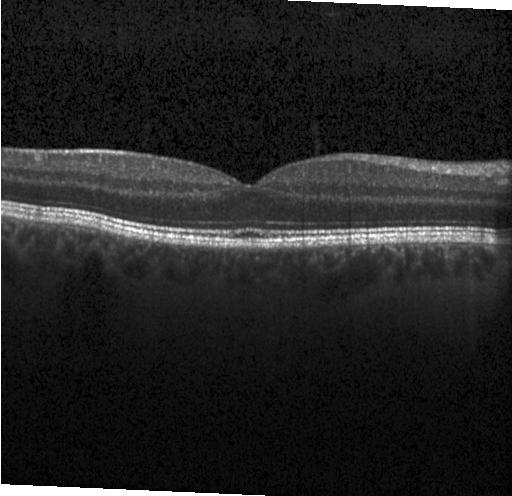 Centered on the fovea, spectral-domain OCT, retinal OCT B-scan.
Impression: no choroidal neovascularization, diabetic macular edema, or drusen.